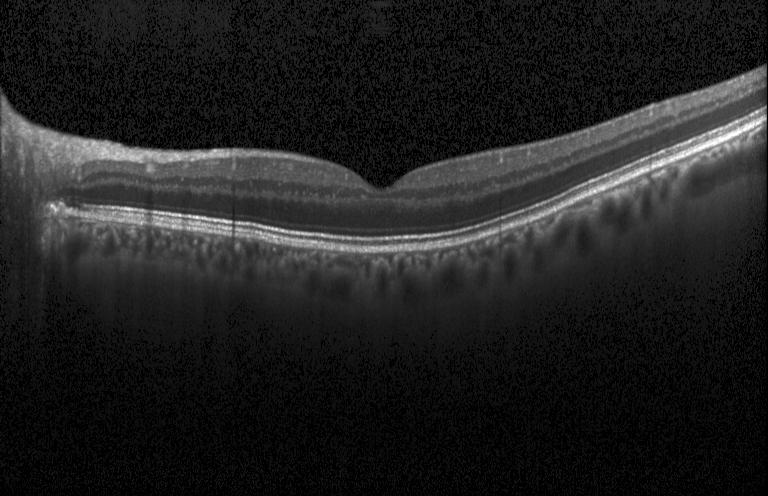
Macular OCT demonstrating no CNV, DME, or drusen.